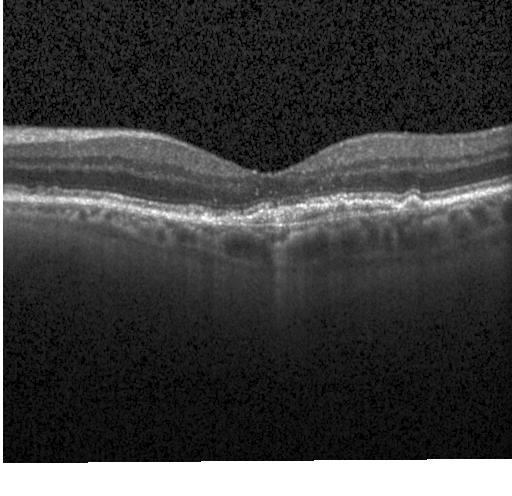
Instrument: Heidelberg Spectralis · macular scan · optical coherence tomography scan.
Impression: choroidal neovascularization.